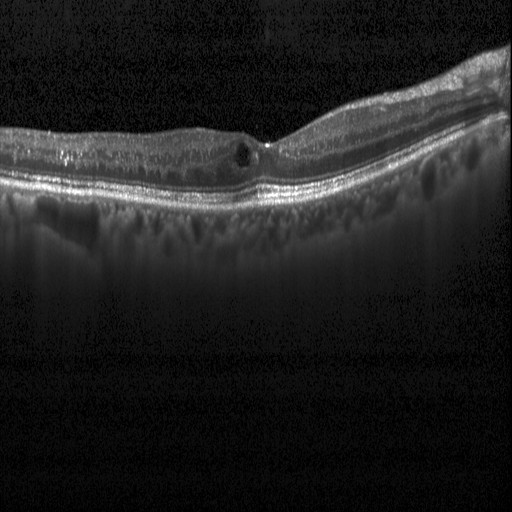

Retinal OCT cross-section.
Diabetic macular edema (DME).